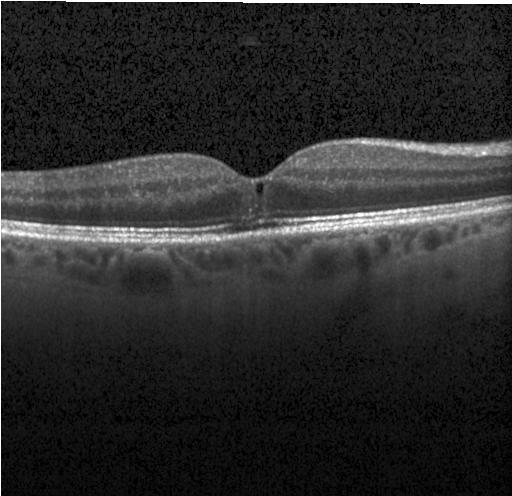

OCT line scan — Impression: diabetic macular edema (DME).